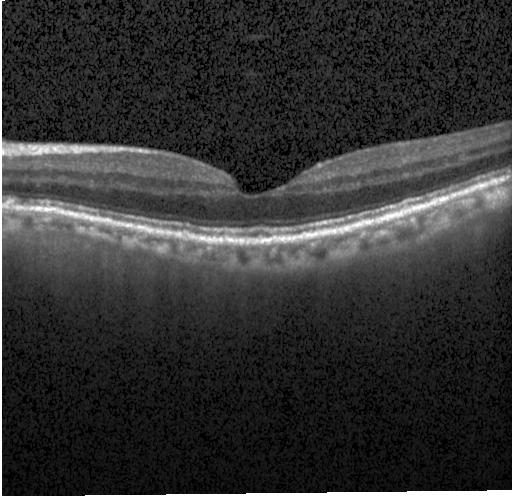

Heidelberg Spectralis · retinal OCT cross-section · macular scan · SD-OCT — Macular OCT: no evidence of CNV, DME, or drusen.